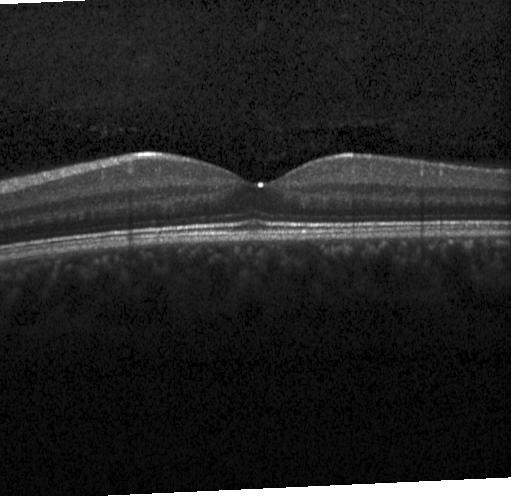

Retinal OCT cross-section
This B-scan demonstrates no choroidal neovascularization, no diabetic macular edema, and no drusen.